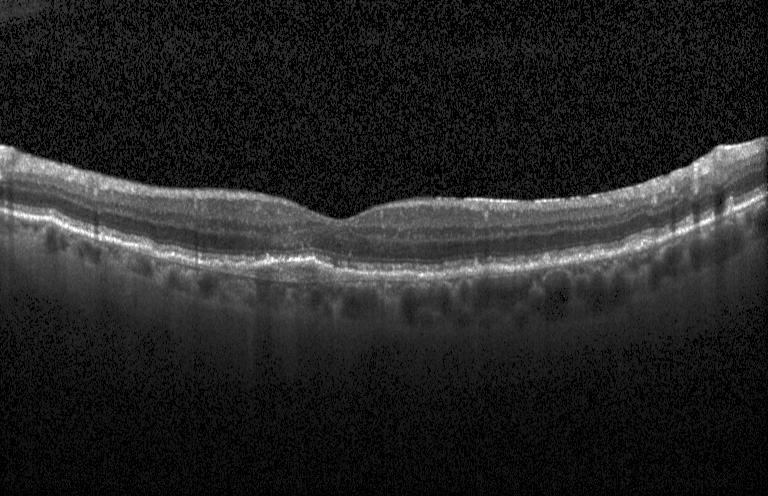
OCT line scan, acquired on a Heidelberg Spectralis
The scan shows choroidal neovascularization.